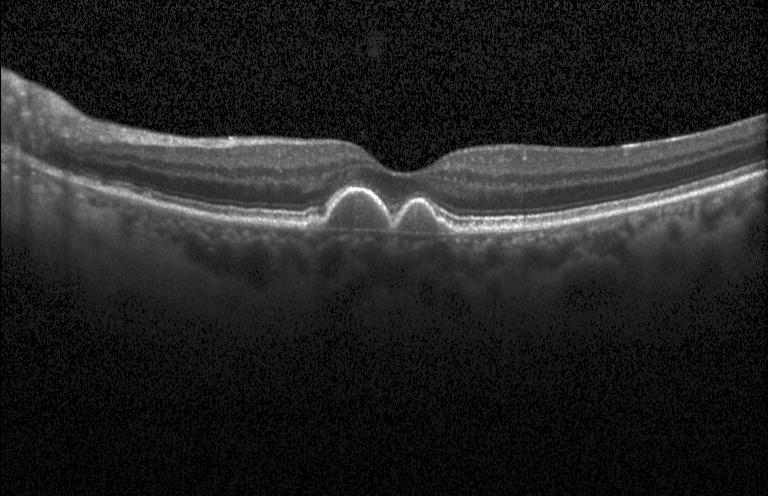 Dx: multiple drusen.